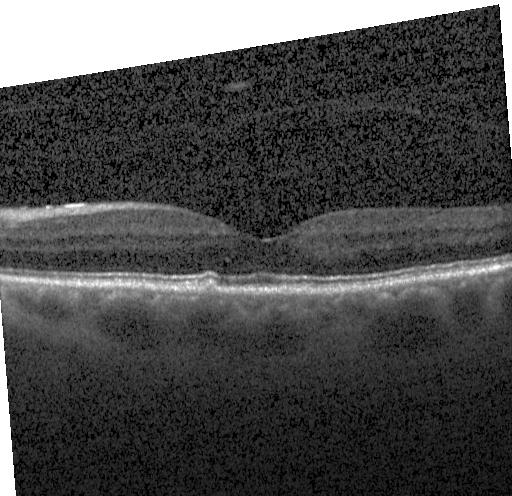
OCT line scan; instrument: Heidelberg Spectralis
Assessment: sub-RPE drusenoid deposits.